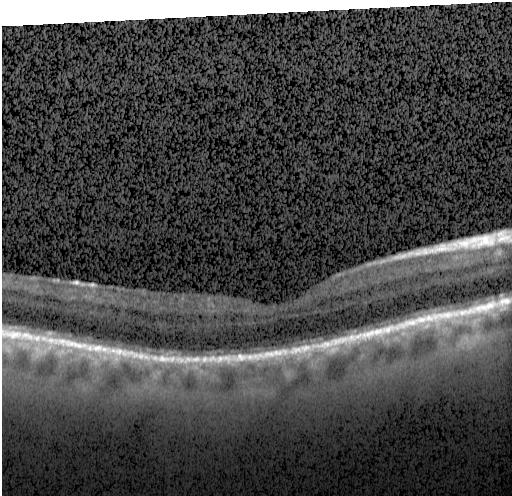

Finding: neither choroidal neovascularization, diabetic macular edema, nor drusen.